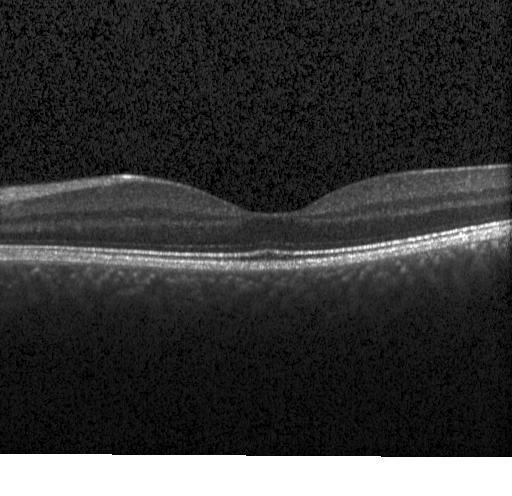 Retinal OCT cross-section.
The scan shows no choroidal neovascularization, no diabetic macular edema, and no drusen.